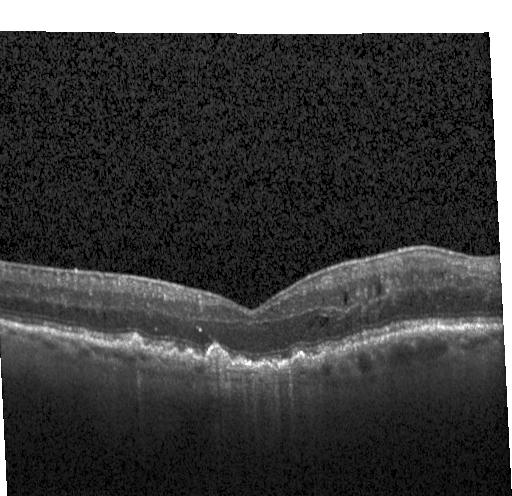

The scan shows a choroidal neovascular membrane.